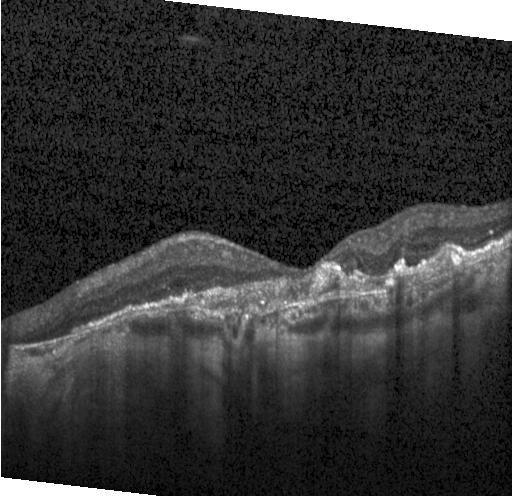 Spectral-domain optical coherence tomography · retinal OCT B-scan — Diagnosis: a choroidal neovascular membrane.